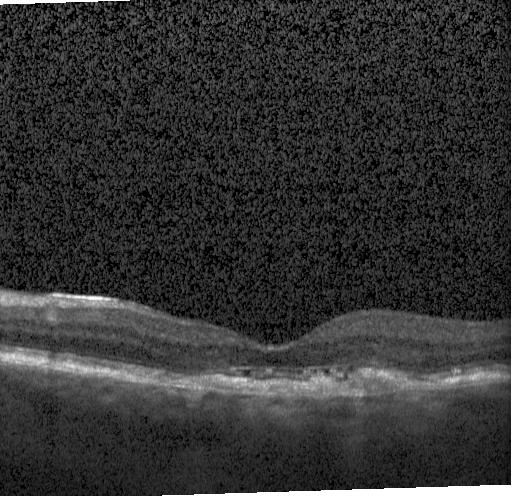
OCT finding: CNV.